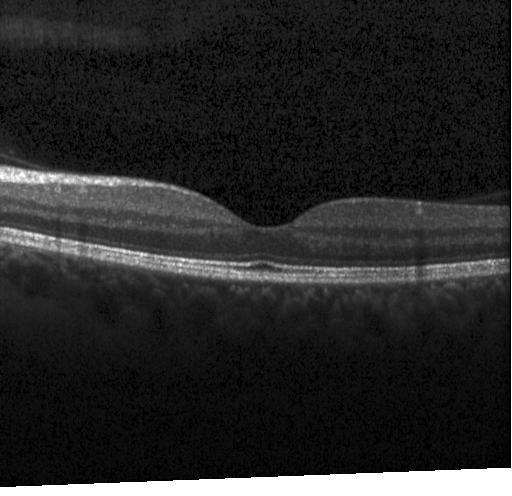

Centered on the fovea. Retinal OCT B-scan. Spectral-domain optical coherence tomography — This B-scan demonstrates neither choroidal neovascularization, diabetic macular edema, nor drusen.